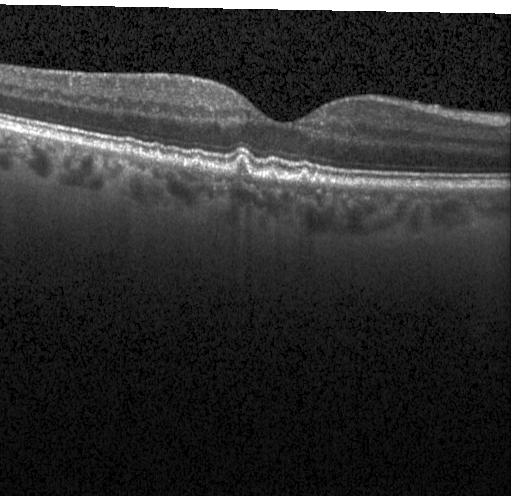 Macular OCT demonstrating sub-RPE drusenoid deposits.